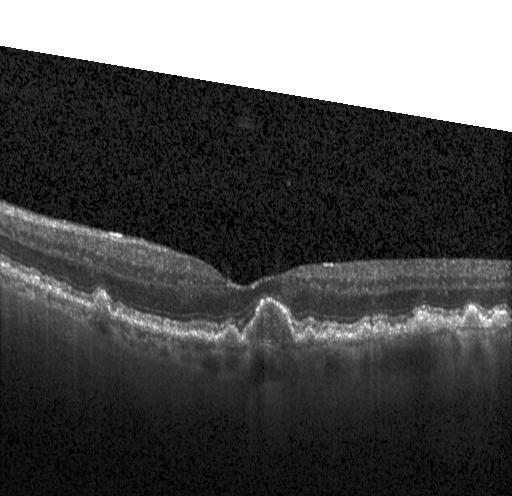 Diagnosis: drusen.